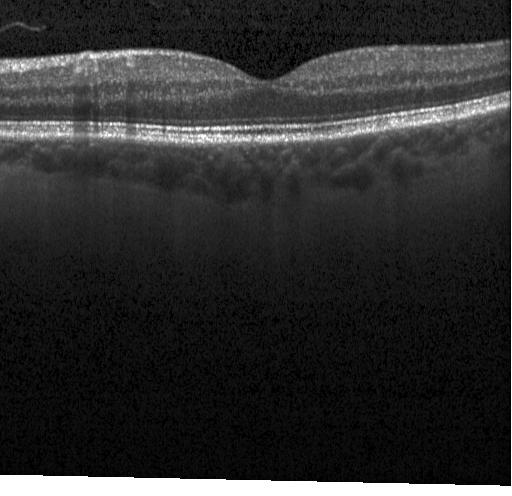 Dx: neither CNV, DME, nor drusen.